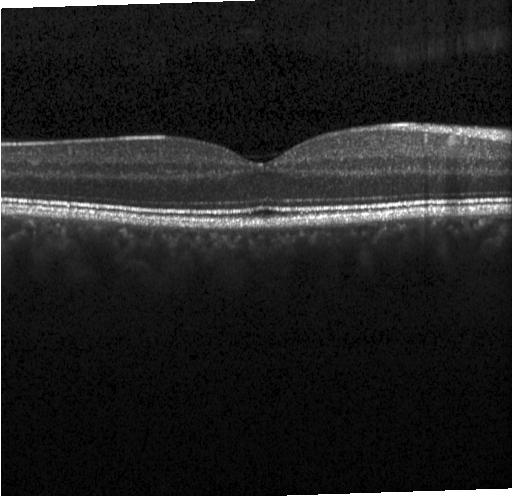

Diagnosis: neither choroidal neovascularization, diabetic macular edema, nor drusen.